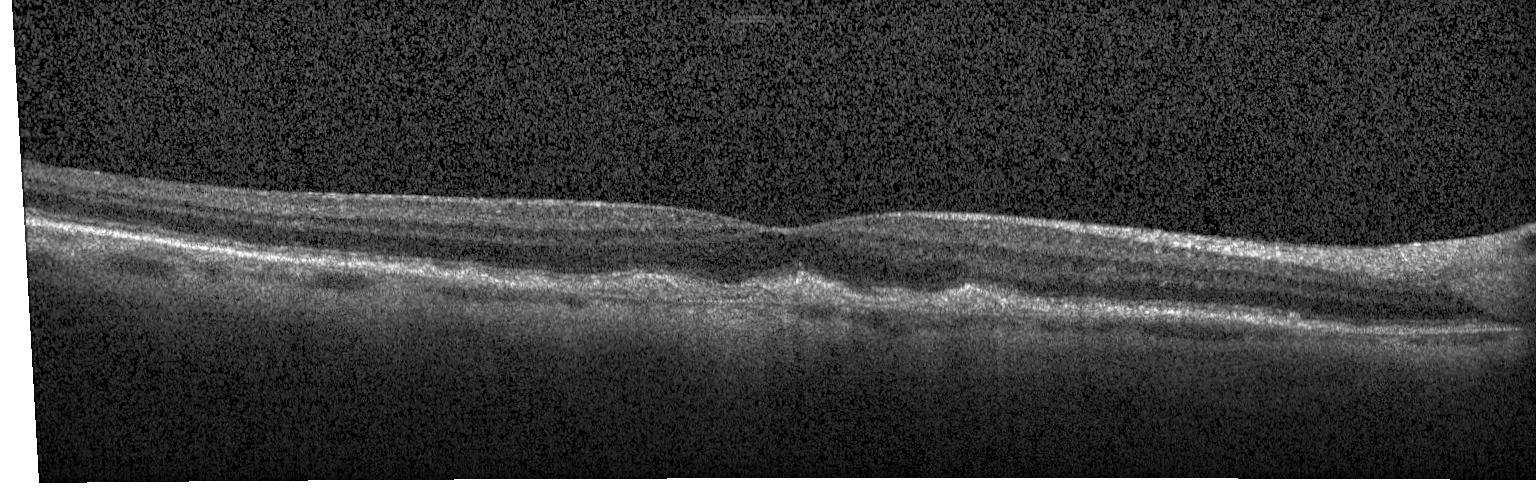 Retinal OCT B-scan. Dx: a choroidal neovascular membrane.